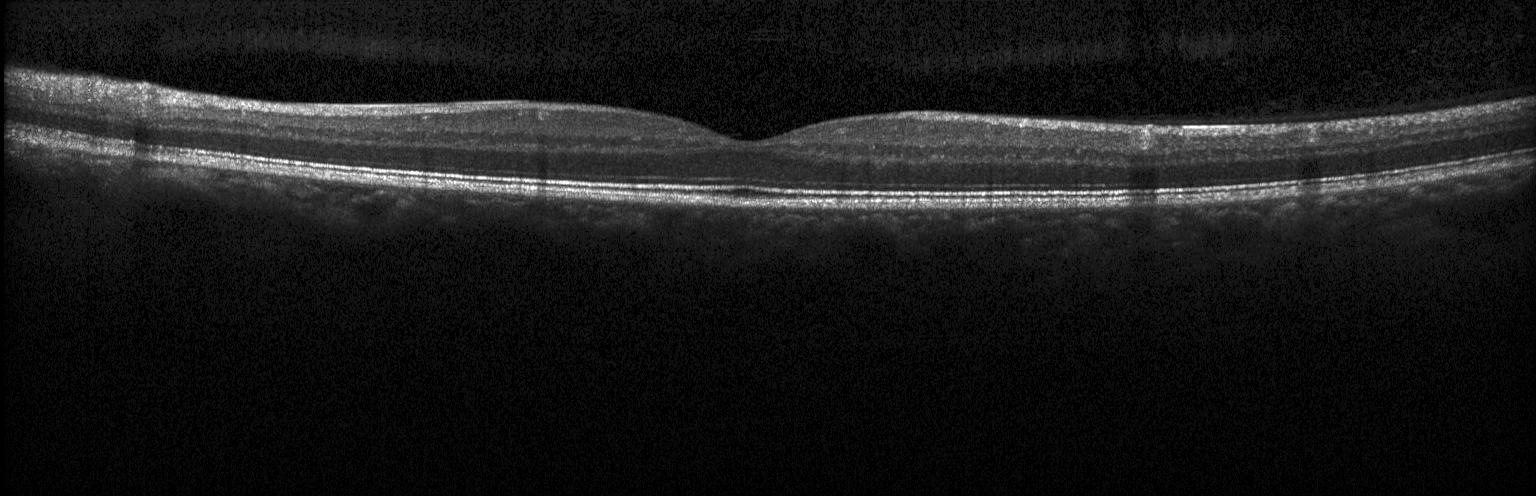
Macular OCT: no evidence of choroidal neovascularization, diabetic macular edema, or drusen.